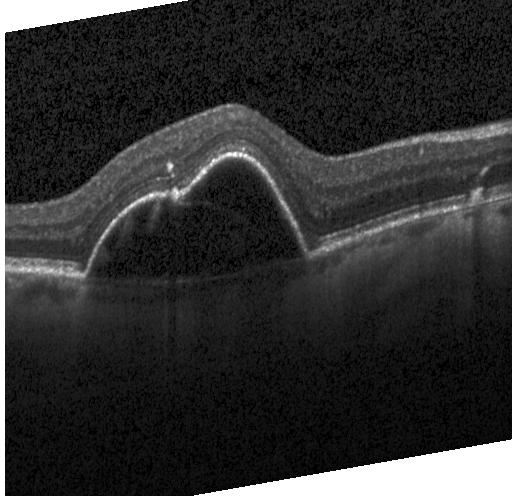 Macular OCT demonstrating a choroidal neovascular membrane.